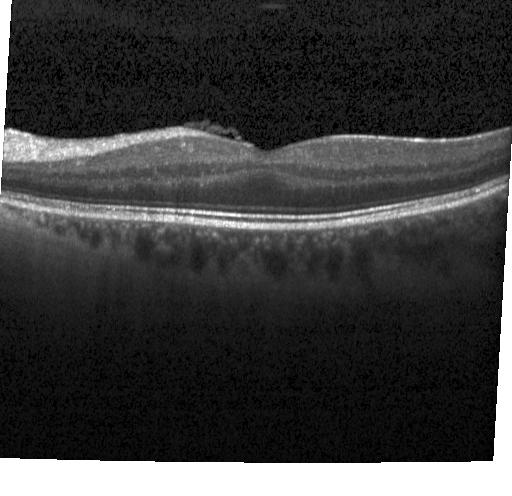
Heidelberg Spectralis OCT system. Centered on the fovea. Spectral-domain OCT. Retinal OCT B-scan. OCT finding: no choroidal neovascularization, diabetic macular edema, or drusen.